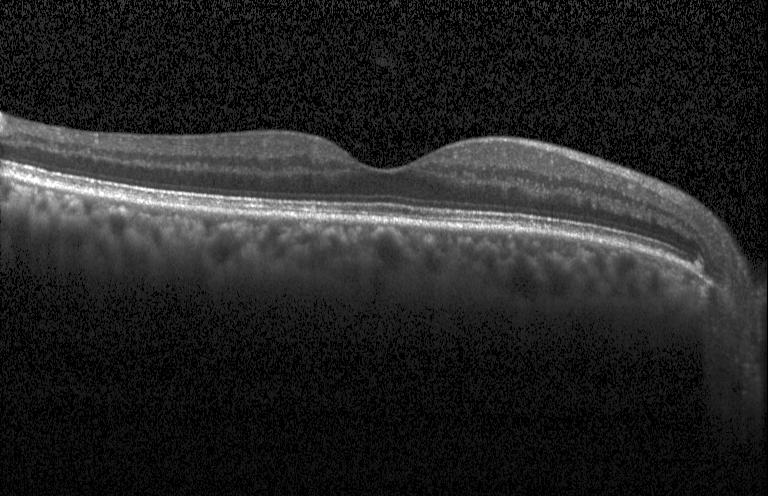

Optical coherence tomography B-scan — Finding: neither choroidal neovascularization, diabetic macular edema, nor drusen.